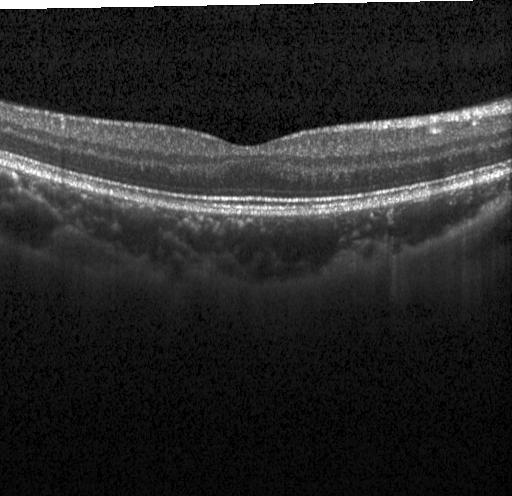

Instrument: Heidelberg Spectralis, retinal OCT B-scan, macular scan, spectral-domain OCT — Impression: neither CNV, DME, nor drusen.